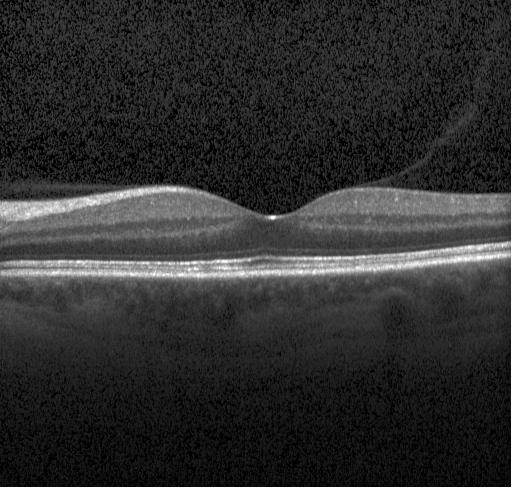 Dx: no choroidal neovascularization, diabetic macular edema, or drusen.